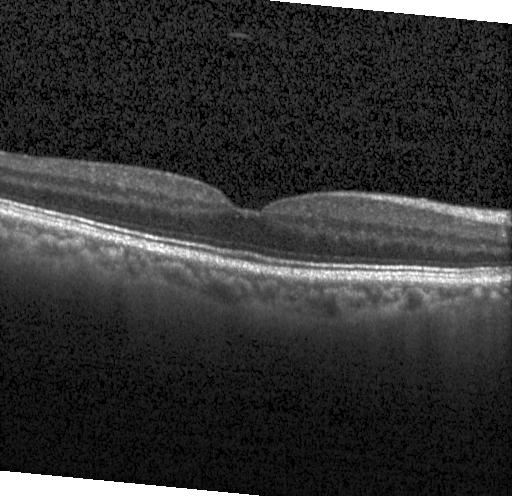

No evidence of CNV, DME, or drusen.